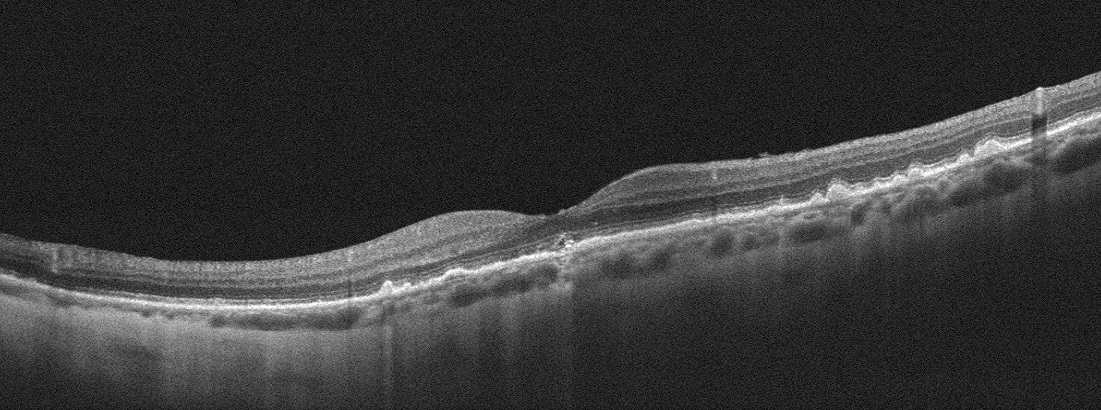 This B-scan demonstrates AMD.